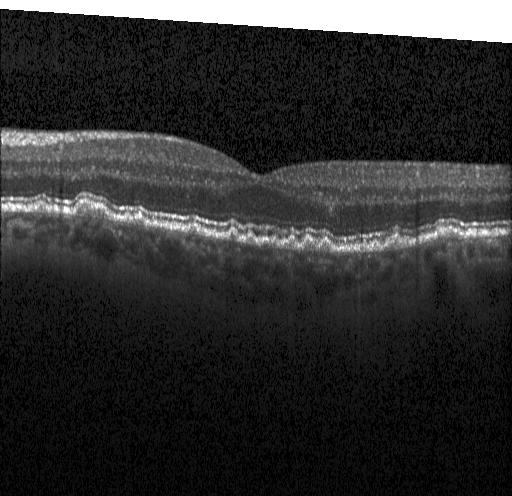

This B-scan demonstrates multiple drusen.